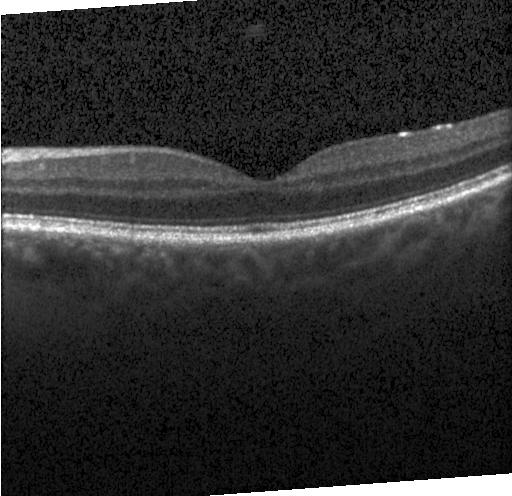

Impression: no CNV, no DME, and no drusen.